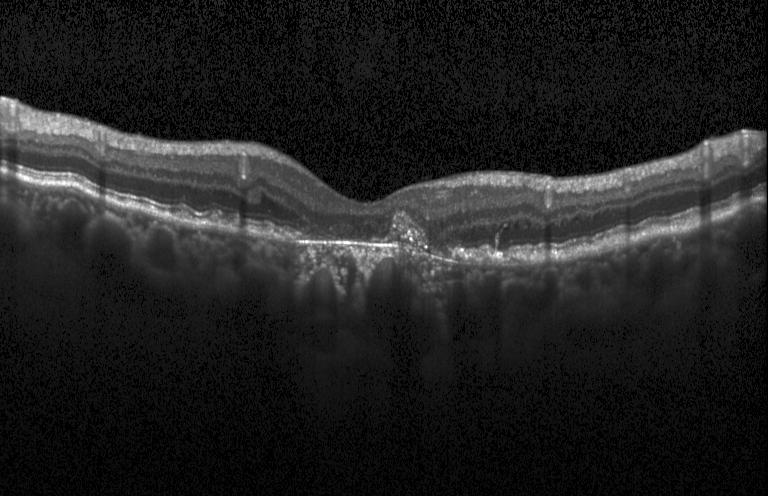
Optical coherence tomography scan · Heidelberg Spectralis OCT system
Impression: CNV.